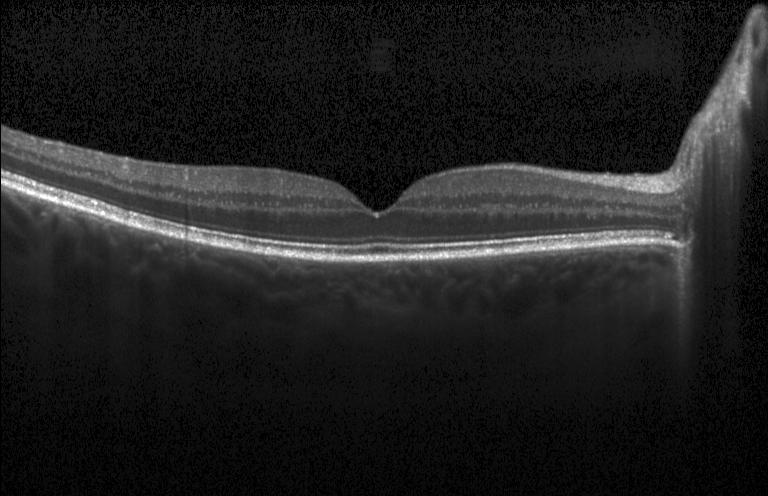
The scan shows no CNV, no DME, and no drusen.